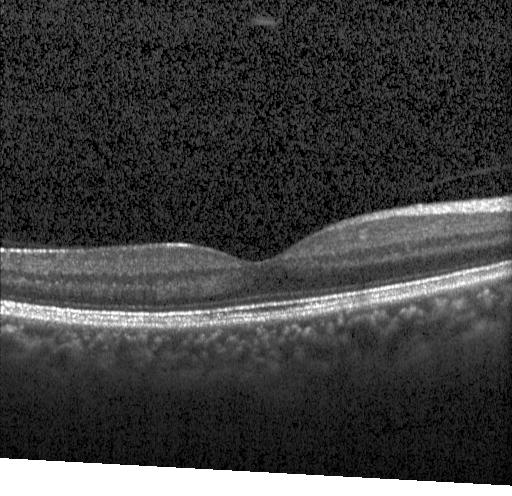 Retinal OCT cross-section, instrument: Heidelberg Spectralis, spectral-domain OCT. Impression: no CNV, no DME, and no drusen.